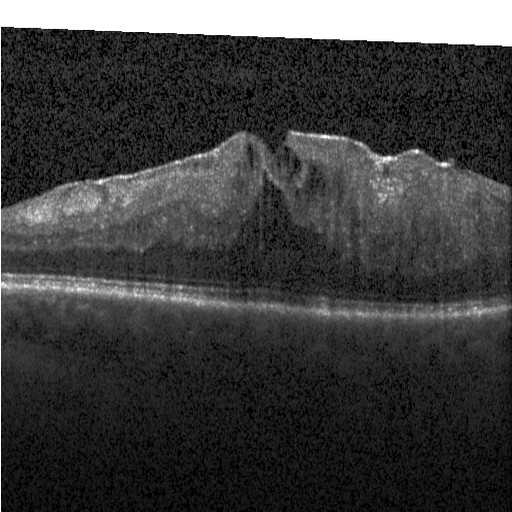
OCT finding: diabetic macular edema (DME).